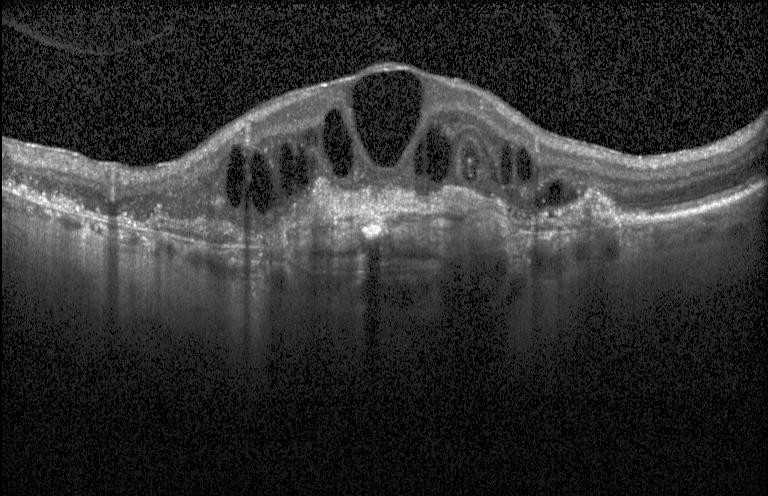

Finding: a choroidal neovascular membrane.